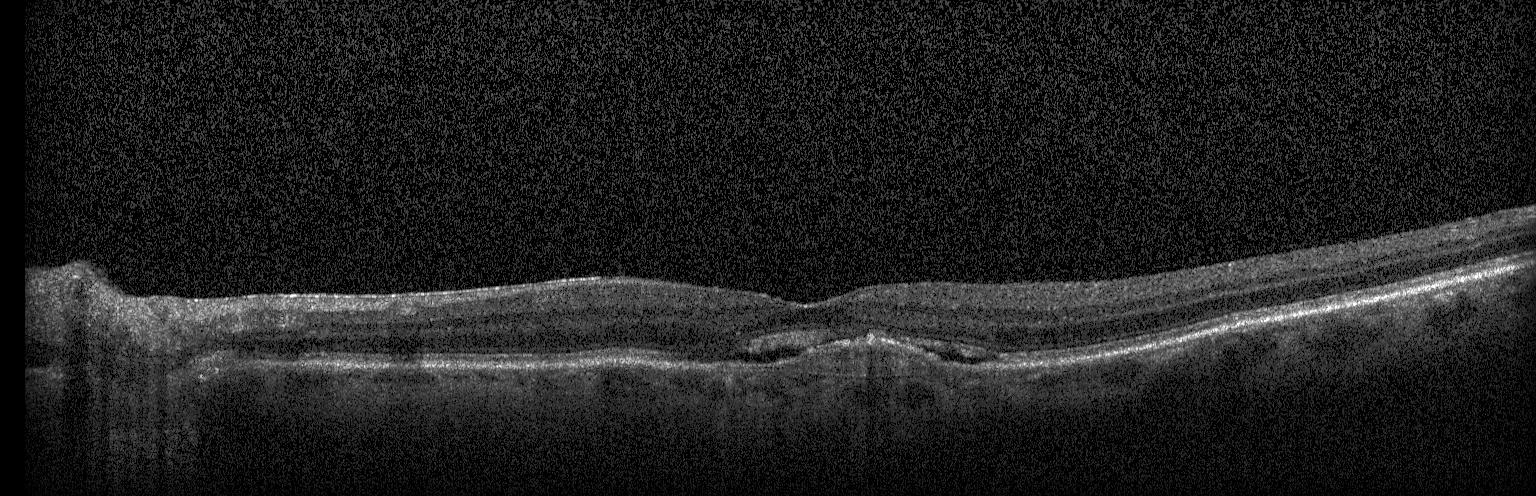
OCT B-scan showing choroidal neovascularization.